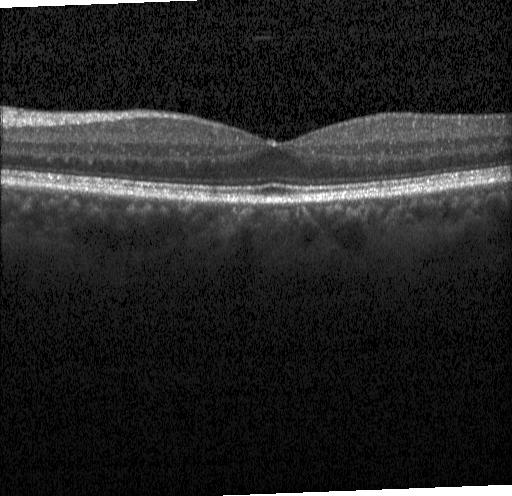

Horizontal scan through the fovea; Heidelberg Spectralis; optical coherence tomography scan; spectral-domain OCT.
Diagnosis: neither CNV, DME, nor drusen.